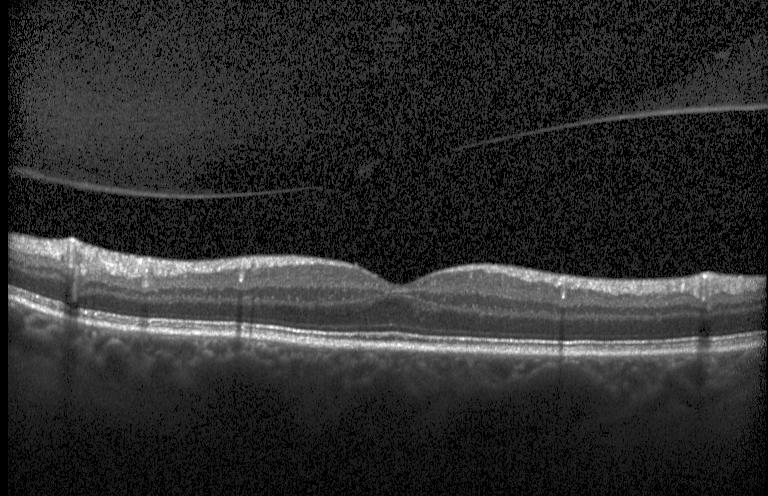
Retinal OCT cross-section, spectral-domain optical coherence tomography, fovea-centered. Impression: no choroidal neovascularization, no diabetic macular edema, and no drusen.